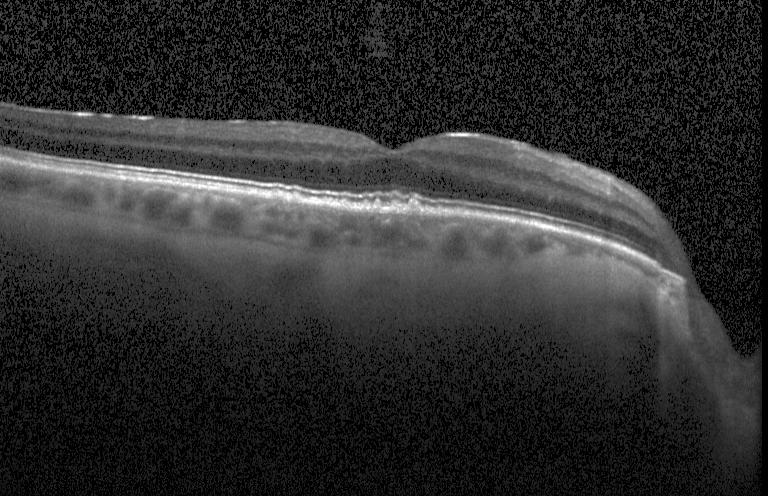 Diagnosis: sub-RPE drusenoid deposits.